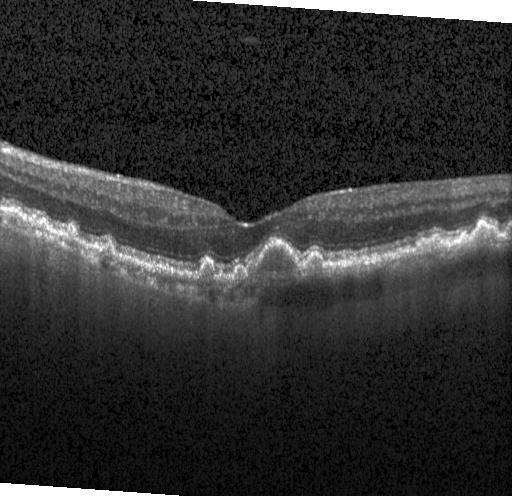
Centered on the fovea · retinal OCT B-scan
Sub-RPE drusenoid deposits.